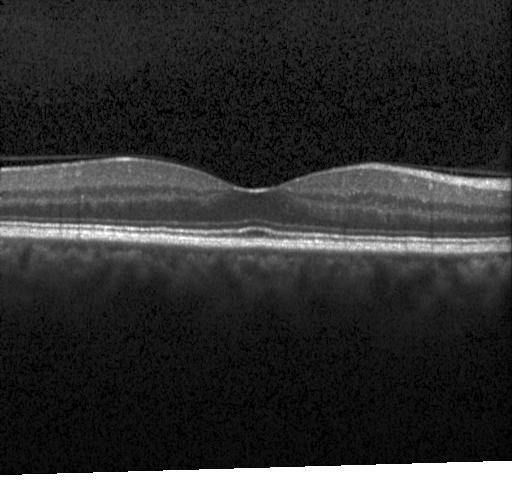

Macular OCT: no choroidal neovascularization, diabetic macular edema, or drusen.